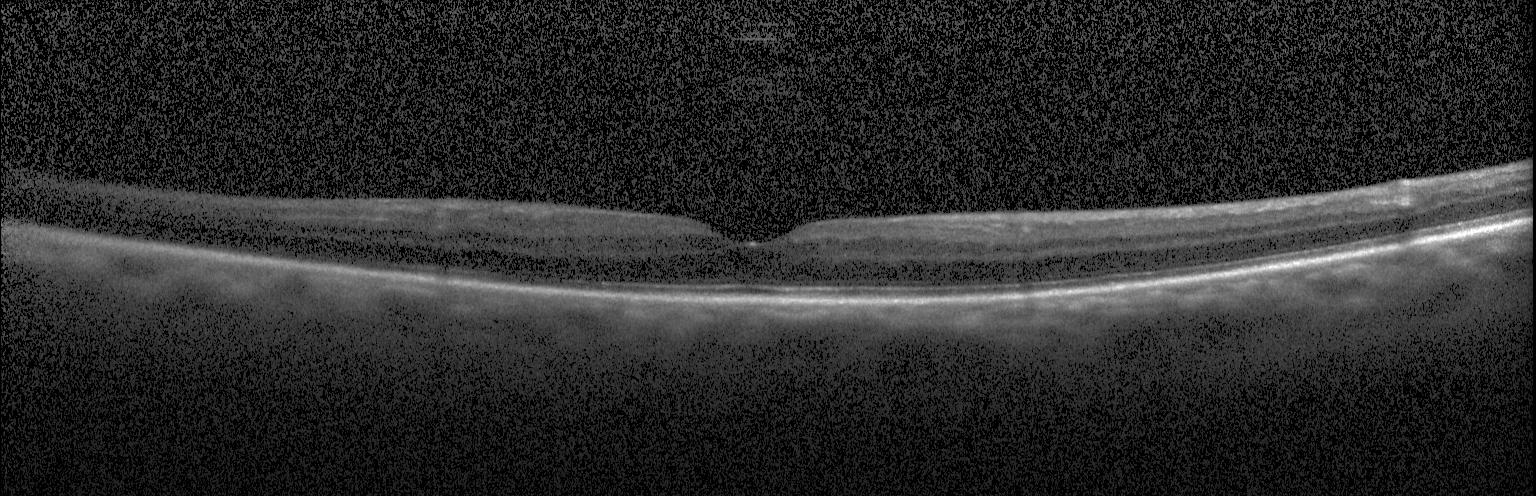

Macular OCT demonstrating no choroidal neovascularization, no diabetic macular edema, and no drusen.